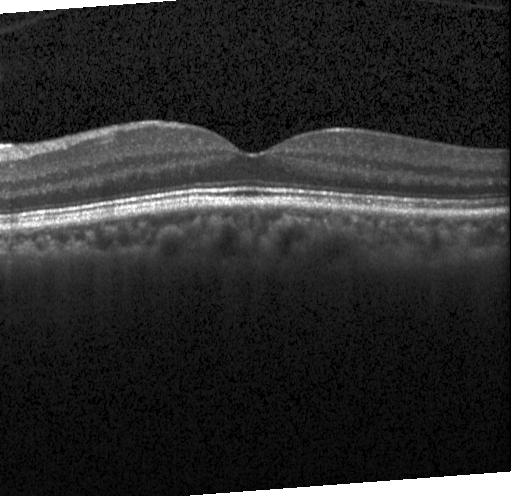 Retinal OCT B-scan. Heidelberg Spectralis. Fovea-centered — The scan shows neither choroidal neovascularization, diabetic macular edema, nor drusen.